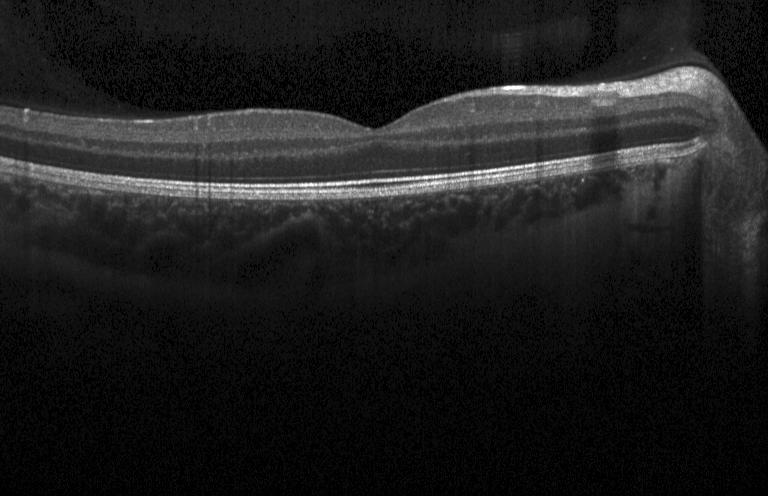 Diagnosis: no CNV, no DME, and no drusen.